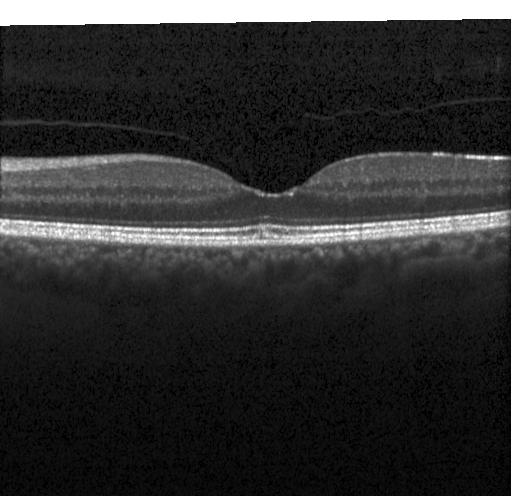
Optical coherence tomography B-scan. Macular scan
Macular OCT: neither CNV, DME, nor drusen.